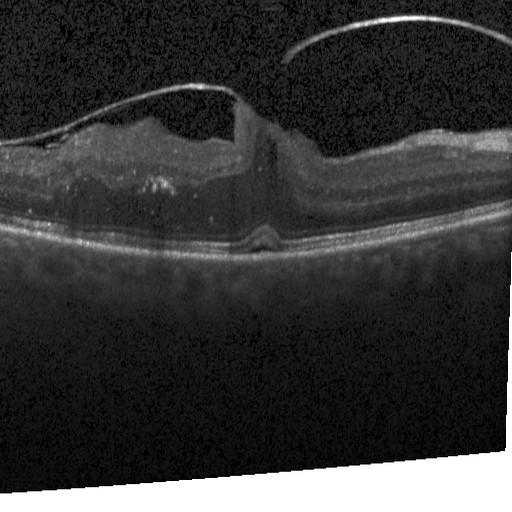

SD-OCT, OCT B-scan — The scan shows DME.